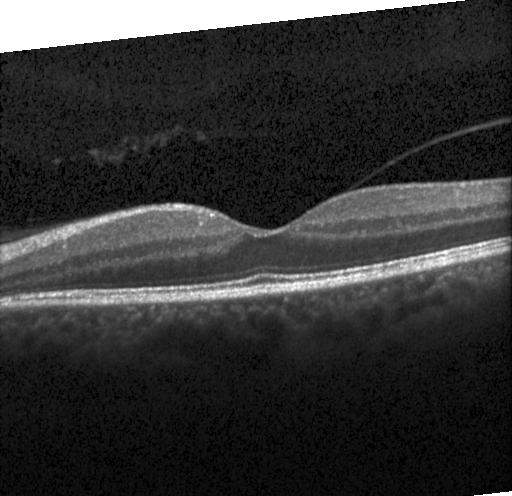 OCT line scan. Diagnosis: no choroidal neovascularization, no diabetic macular edema, and no drusen.